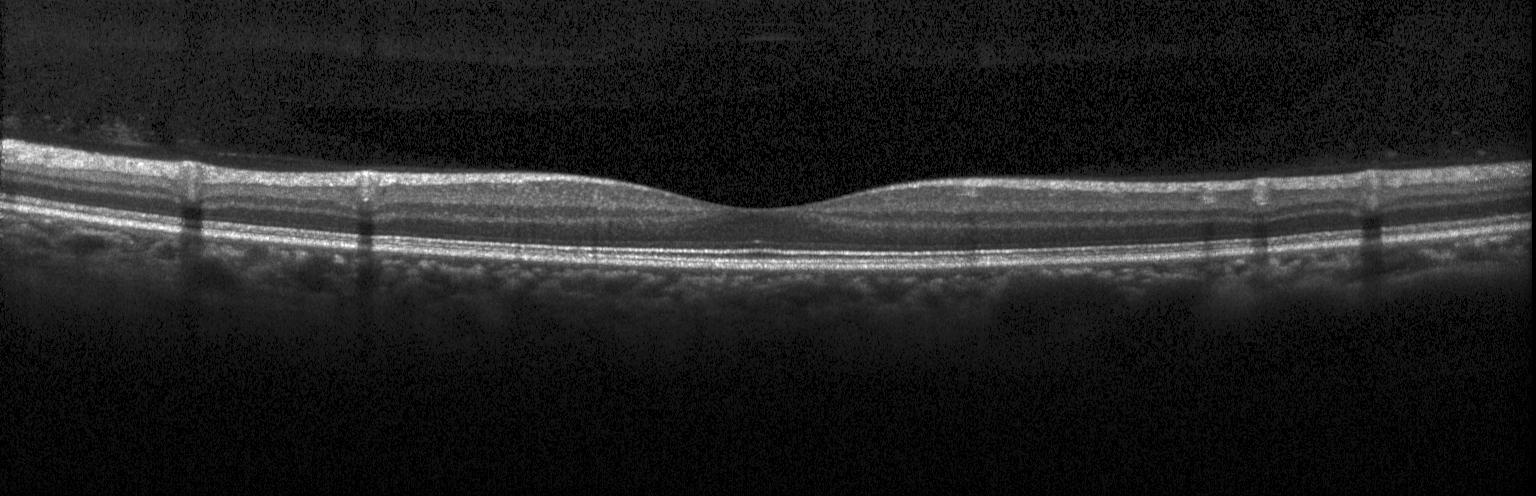 OCT line scan · horizontal scan through the fovea. Impression: neither choroidal neovascularization, diabetic macular edema, nor drusen.